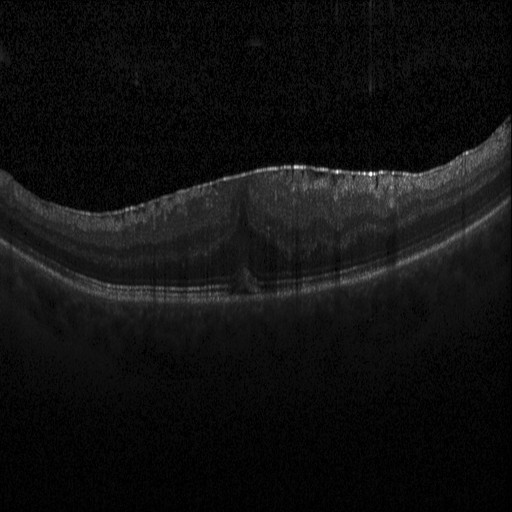
Macular OCT: DME.